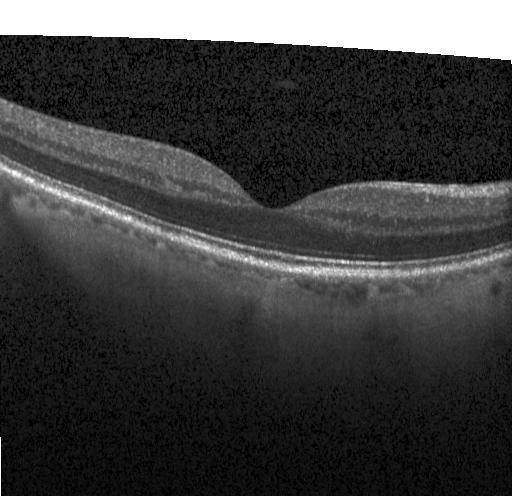 Spectral-domain OCT · retinal OCT B-scan · instrument: Heidelberg Spectralis — Assessment: no CNV, no DME, and no drusen.